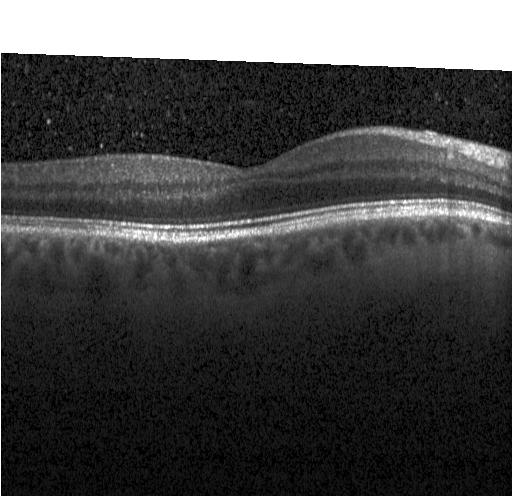
Centered on the fovea · Heidelberg Spectralis OCT system · SD-OCT · OCT B-scan — Finding: neither choroidal neovascularization, diabetic macular edema, nor drusen.